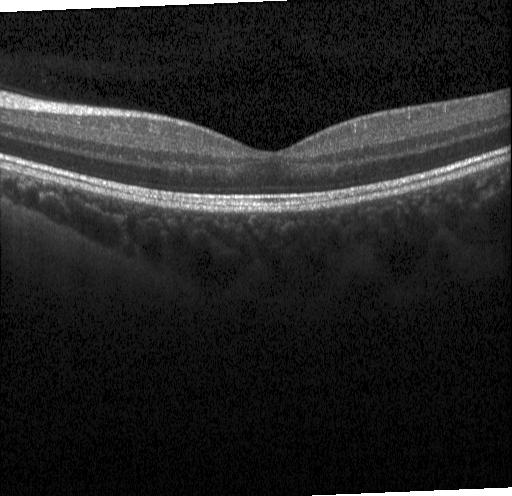

Finding: no choroidal neovascularization, no diabetic macular edema, and no drusen.